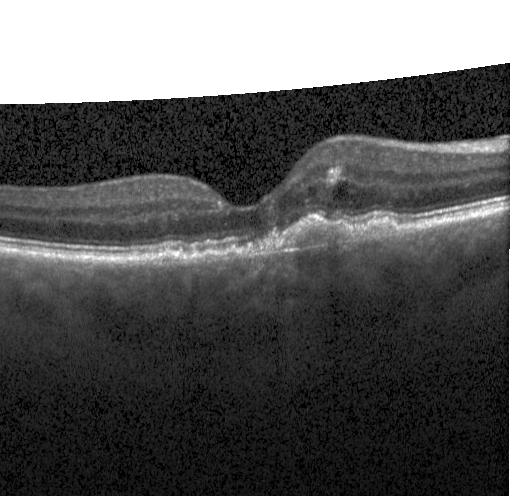

Heidelberg Spectralis OCT system. OCT line scan. Centered on the fovea. Finding: choroidal neovascularization (CNV).